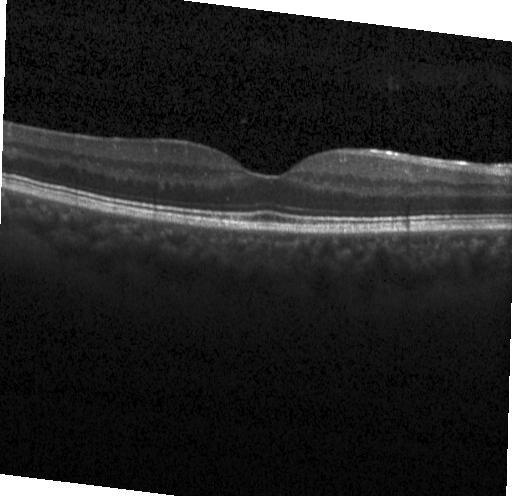
Optical coherence tomography scan · centered on the fovea · spectral-domain optical coherence tomography. Impression: no choroidal neovascularization, no diabetic macular edema, and no drusen.